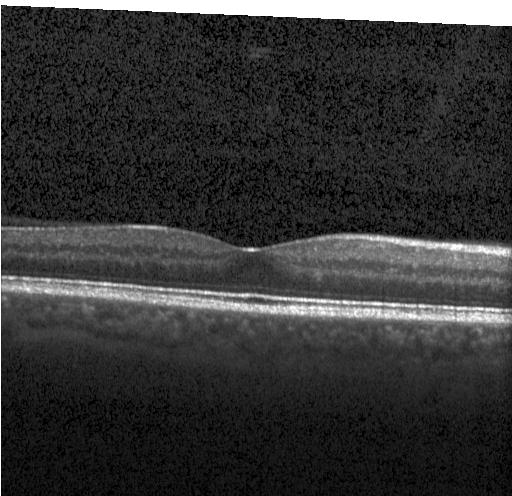

Retinal OCT cross-section showing neither choroidal neovascularization, diabetic macular edema, nor drusen.